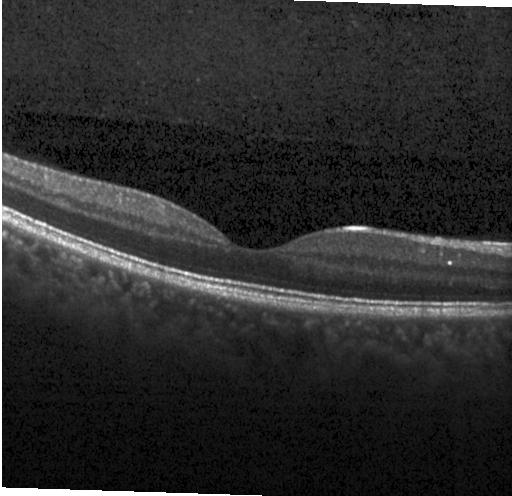
Horizontal scan through the fovea · optical coherence tomography B-scan · Heidelberg Spectralis
Macular OCT: no choroidal neovascularization, diabetic macular edema, or drusen.